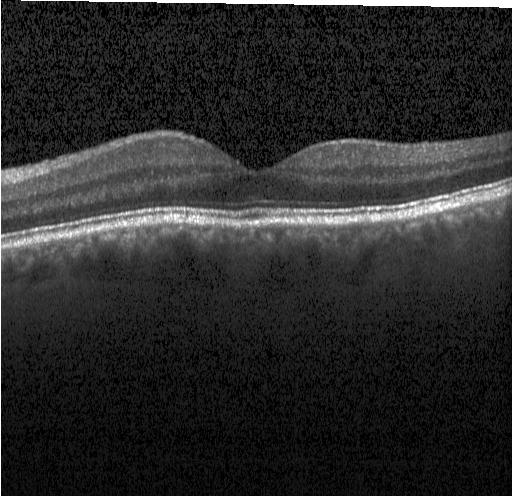 Impression: no CNV, DME, or drusen.